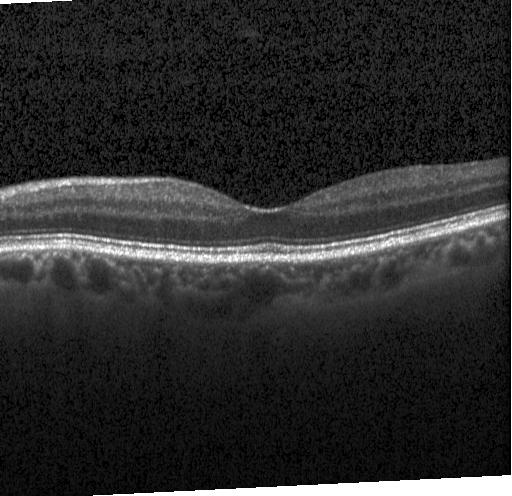

Spectral-domain optical coherence tomography, horizontal scan through the fovea, optical coherence tomography B-scan, Heidelberg Spectralis OCT system.
Impression: no choroidal neovascularization, diabetic macular edema, or drusen.